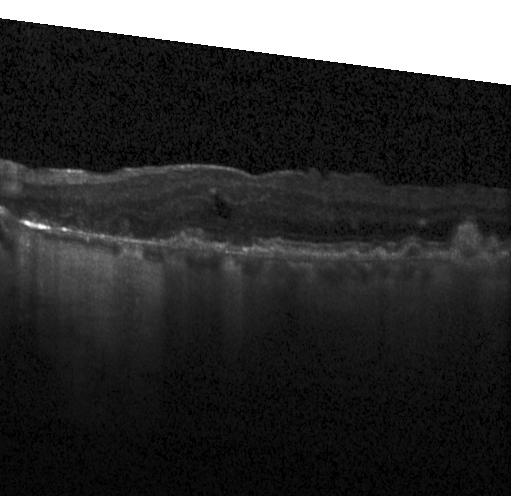

Dx: a choroidal neovascular membrane.